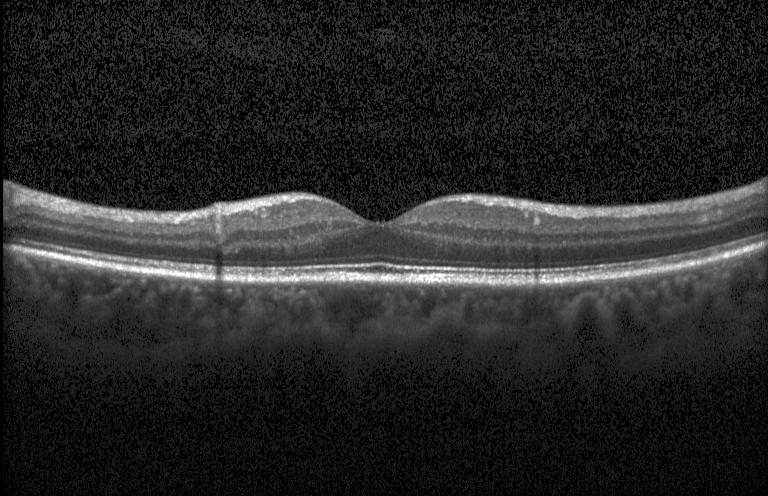 OCT line scan. Finding: neither choroidal neovascularization, diabetic macular edema, nor drusen.